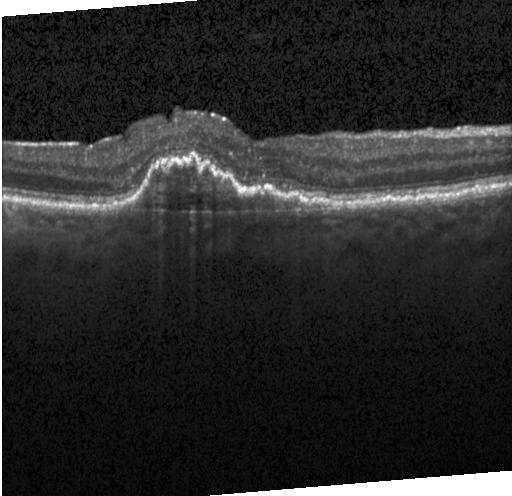
Retinal OCT cross-section — Assessment: a choroidal neovascular membrane.